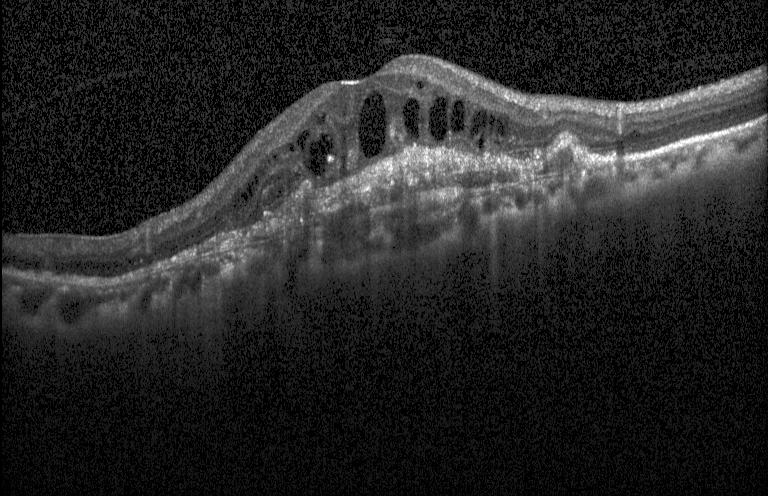 OCT line scan — A choroidal neovascular membrane.